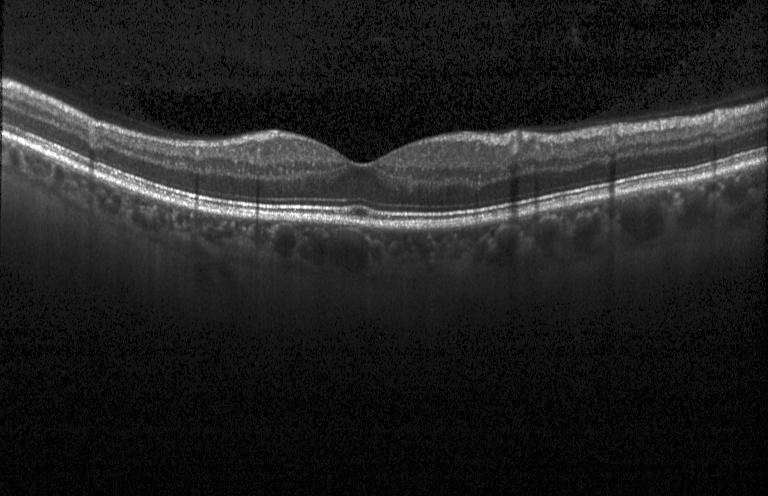
Retinal OCT B-scan, through the macula, instrument: Heidelberg Spectralis, spectral-domain OCT.
No choroidal neovascularization, diabetic macular edema, or drusen.